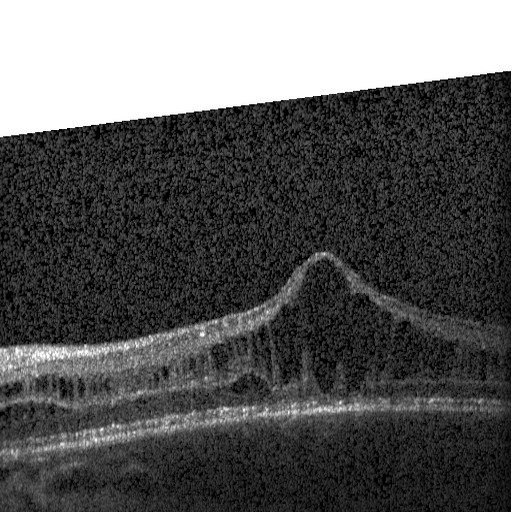

Retinal OCT cross-section showing diabetic macular edema (DME).